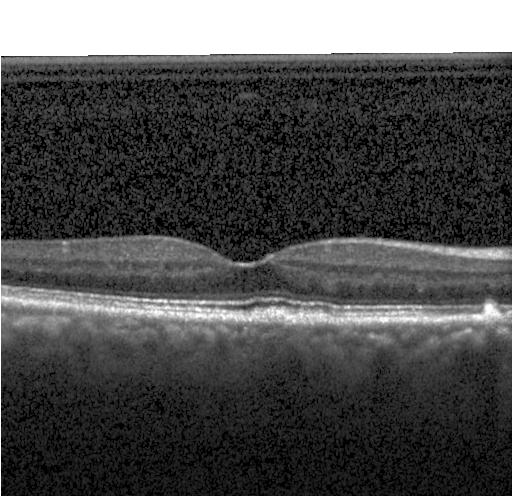 Optical coherence tomography B-scan. Finding: sub-RPE drusenoid deposits.